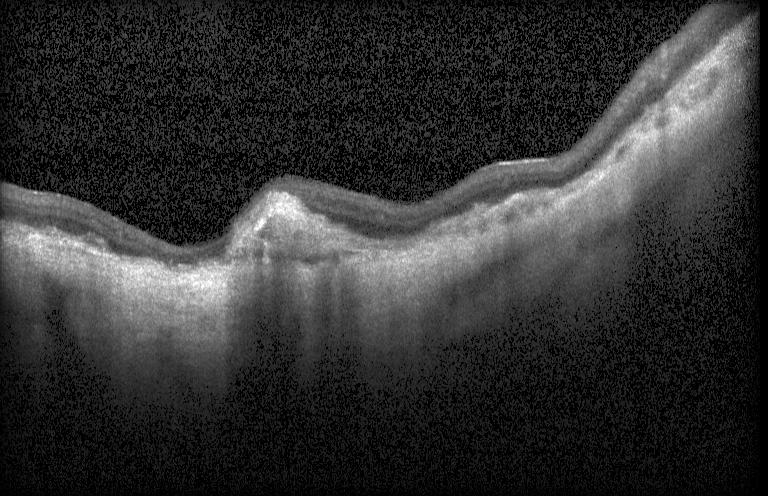 Heidelberg Spectralis; OCT line scan.
This B-scan demonstrates choroidal neovascularization.